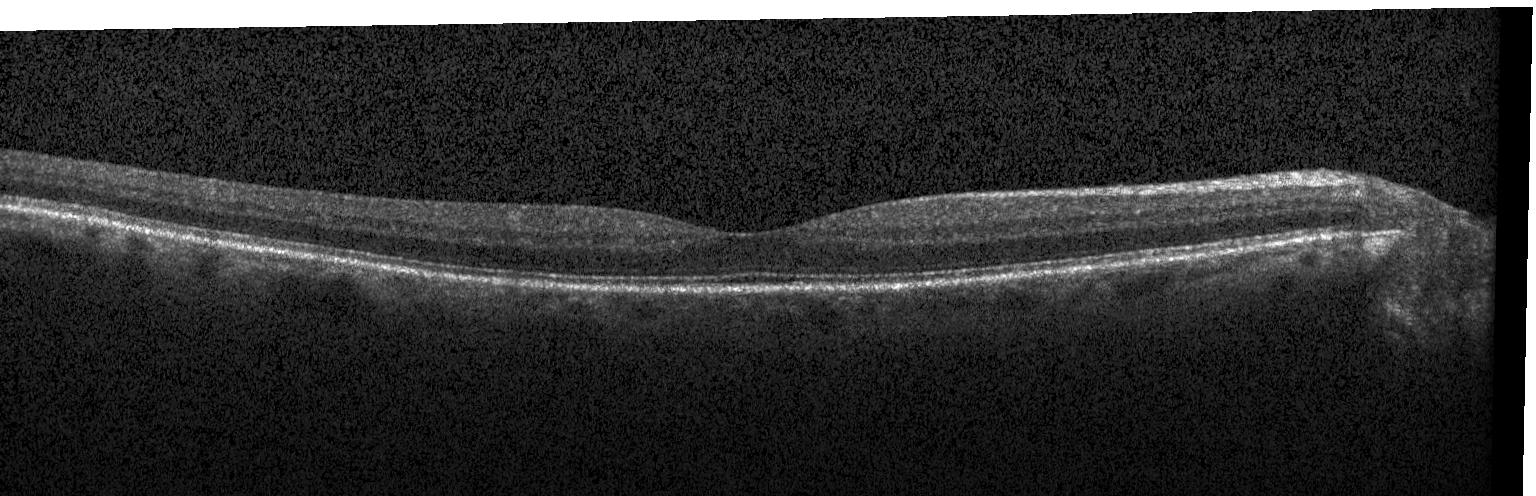

OCT B-scan.
Neither choroidal neovascularization, diabetic macular edema, nor drusen.